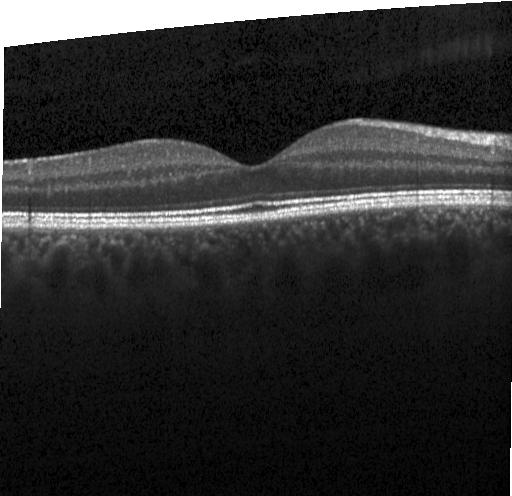

Optical coherence tomography B-scan. Finding: no choroidal neovascularization, diabetic macular edema, or drusen.